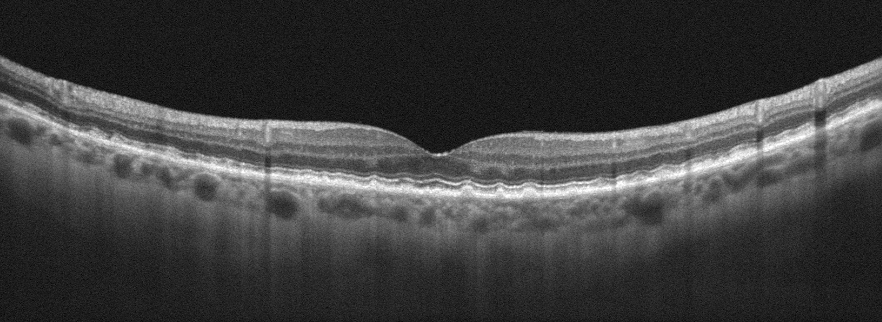
Oculus sinister. OCT B-scan. Assessment: AMD.